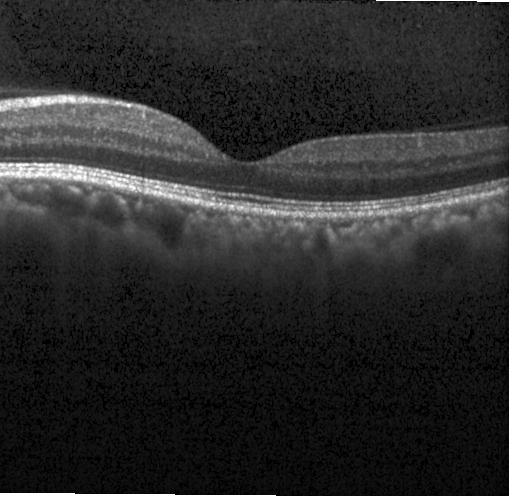
OCT B-scan; spectral-domain OCT; macular scan — Impression: no CNV, no DME, and no drusen.